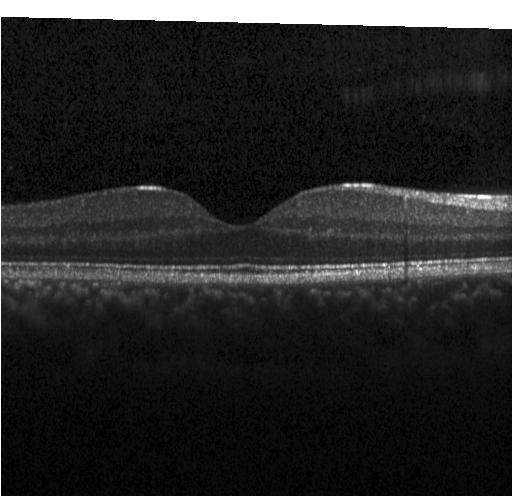 Through the macula · optical coherence tomography scan.
OCT finding: no evidence of choroidal neovascularization, diabetic macular edema, or drusen.